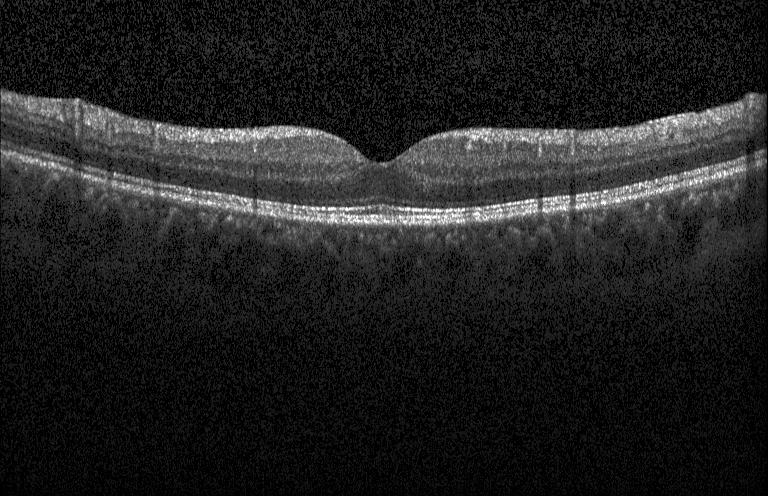 Instrument: Heidelberg Spectralis; OCT B-scan.
Dx: no evidence of choroidal neovascularization, diabetic macular edema, or drusen.